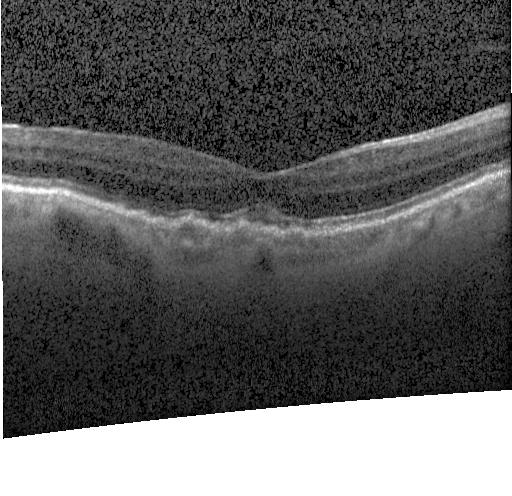

OCT B-scan, fovea-centered, SD-OCT. Finding: CNV.